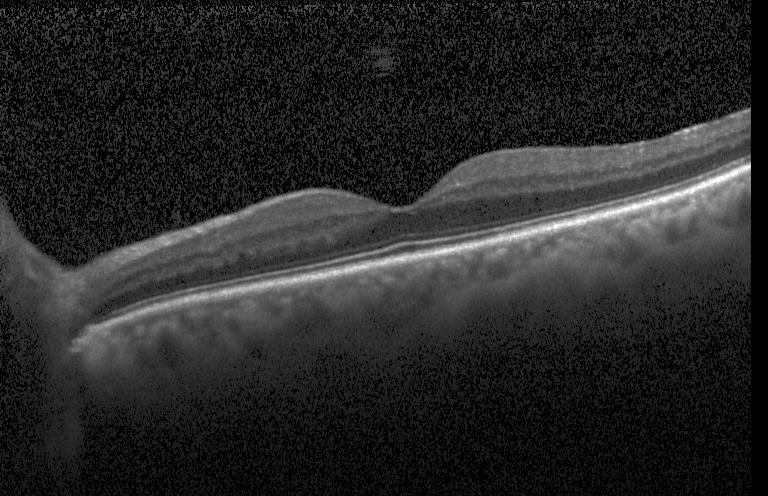 Dx: no choroidal neovascularization, diabetic macular edema, or drusen.